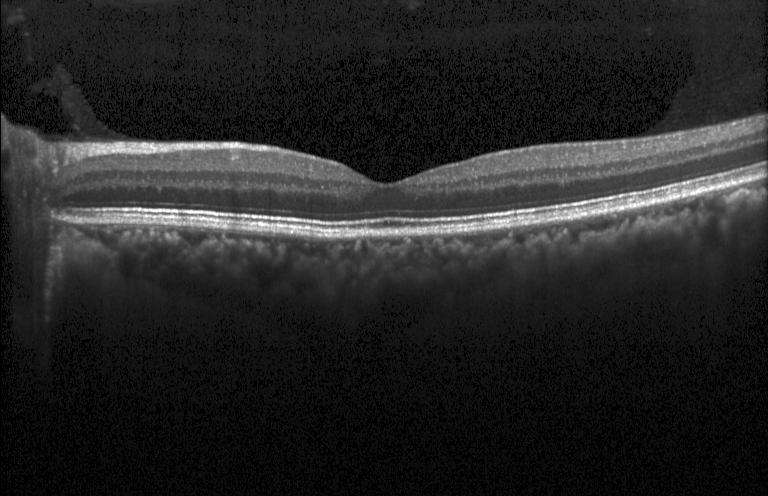 OCT B-scan showing neither choroidal neovascularization, diabetic macular edema, nor drusen.